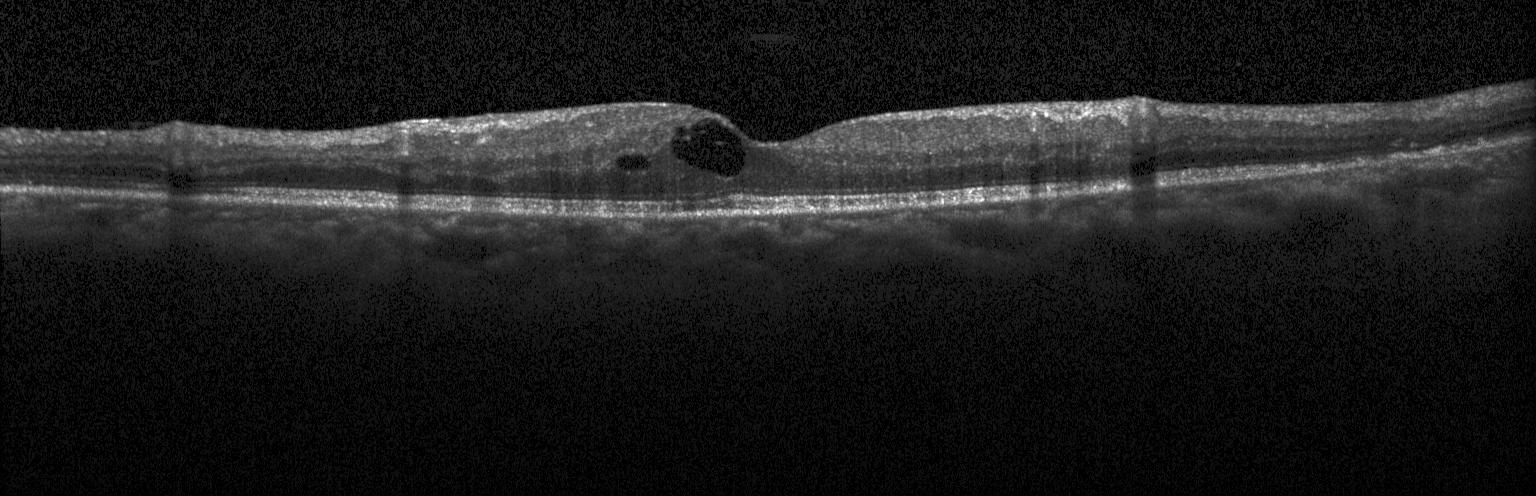

Horizontal scan through the fovea; retinal OCT B-scan; SD-OCT; acquired on a Heidelberg Spectralis.
Assessment: diabetic macular edema (DME).